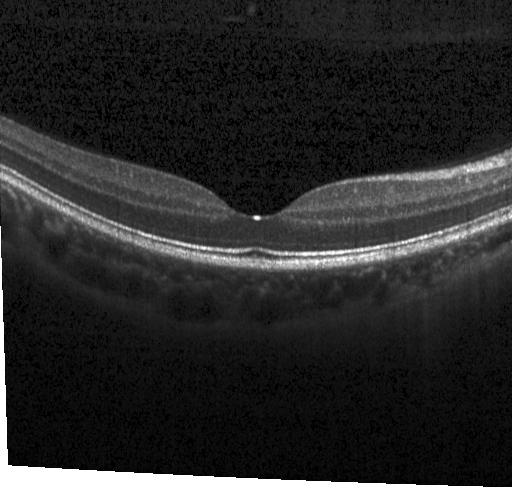
SD-OCT. Optical coherence tomography scan. Instrument: Heidelberg Spectralis. Through the macula. Assessment: no evidence of CNV, DME, or drusen.